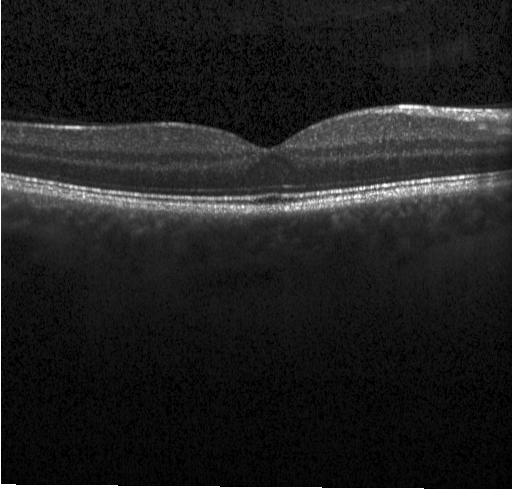
Optical coherence tomography B-scan — OCT finding: no evidence of choroidal neovascularization, diabetic macular edema, or drusen.